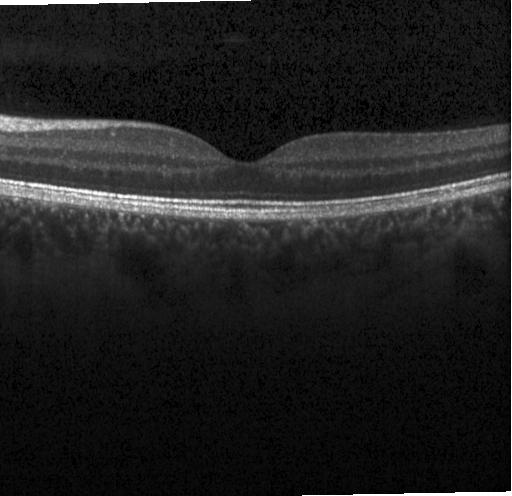 Macular OCT: neither choroidal neovascularization, diabetic macular edema, nor drusen.